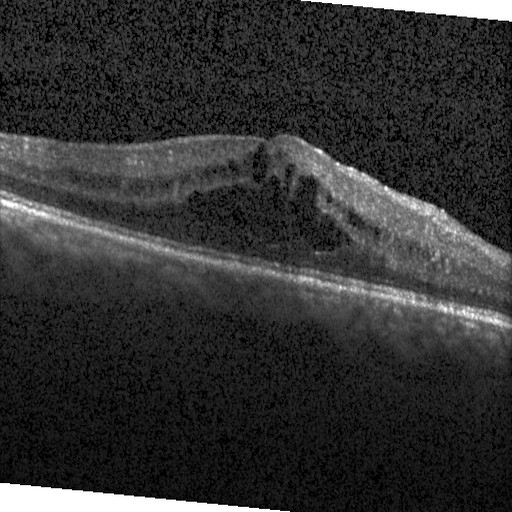
OCT B-scan showing diabetic macular edema (DME).